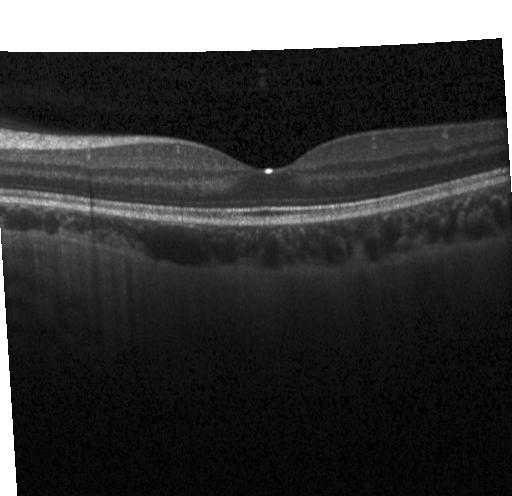
OCT B-scan showing no choroidal neovascularization, no diabetic macular edema, and no drusen.